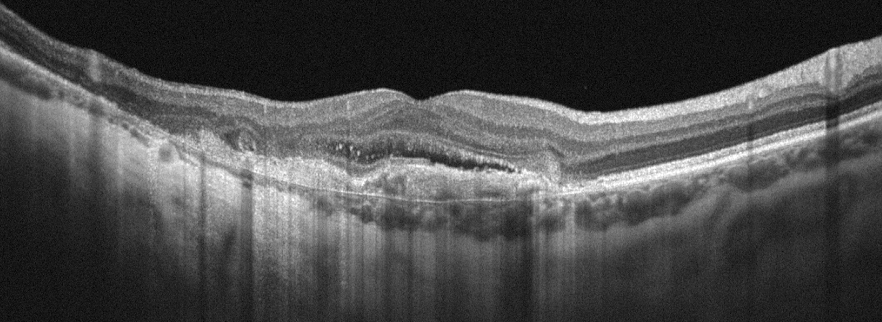

Optical coherence tomography scan · oculus dexter. Assessment: age-related macular degeneration.